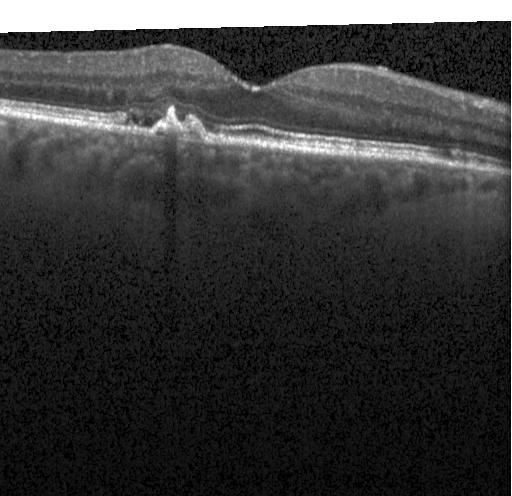

Macular OCT: CNV.